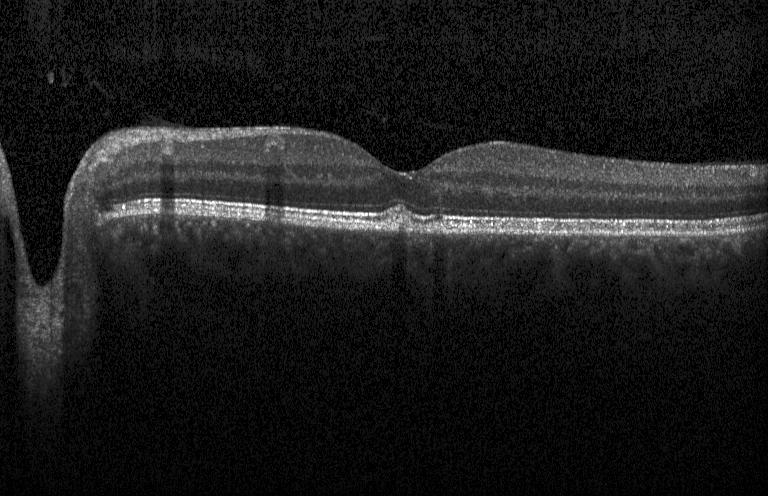

OCT line scan
Finding: sub-RPE drusenoid deposits.